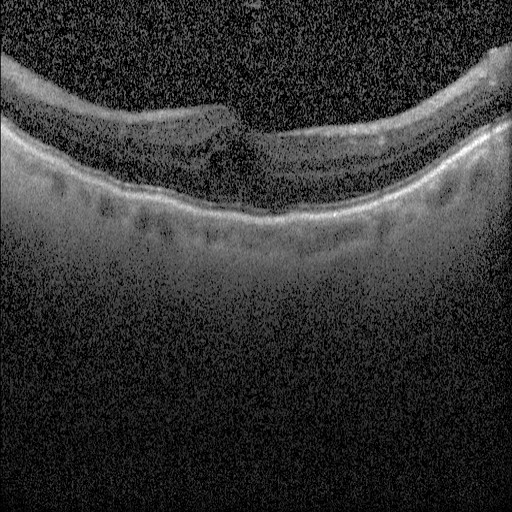 Spectral-domain OCT; retinal OCT B-scan
Dx: DME.